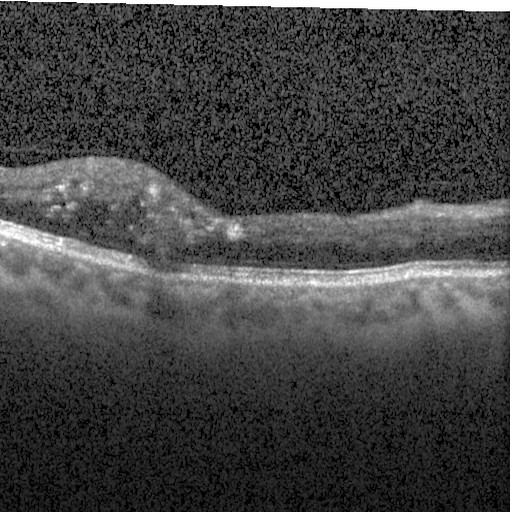

Spectral-domain OCT; OCT line scan; fovea-centered
Diagnosis: diabetic macular edema (DME).